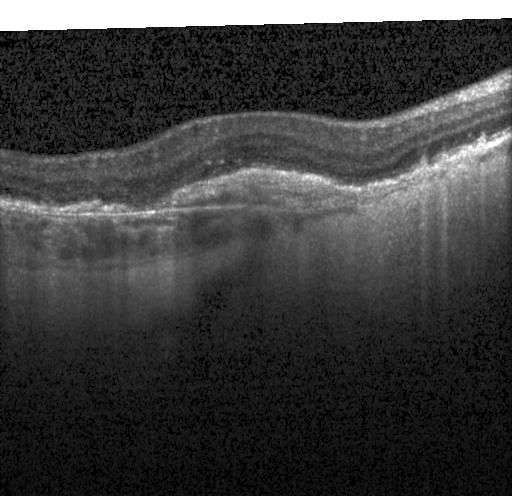

Retinal OCT cross-section
Impression: choroidal neovascularization.